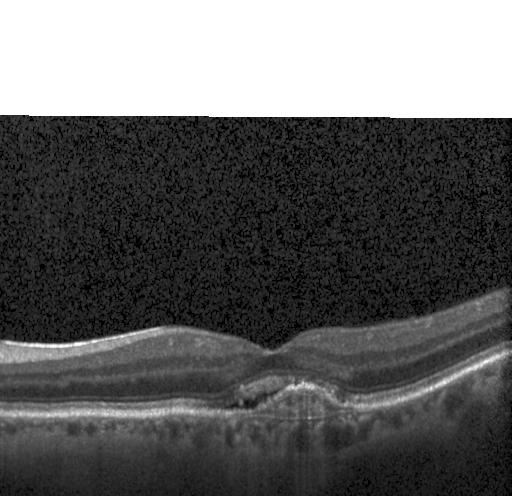 Horizontal scan through the fovea, OCT line scan, spectral-domain OCT, Heidelberg Spectralis OCT system. This B-scan demonstrates CNV.